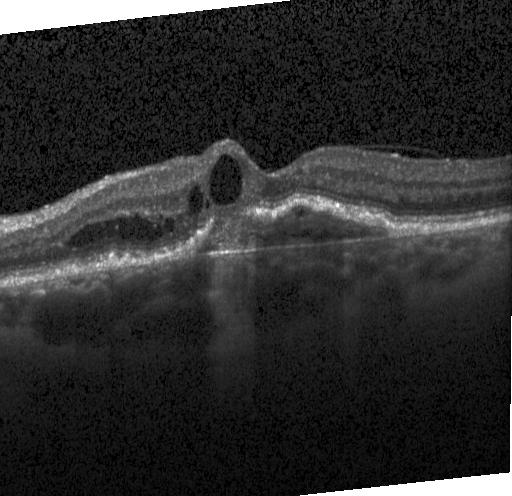
Instrument: Heidelberg Spectralis. OCT B-scan
Diagnosis: choroidal neovascularization.